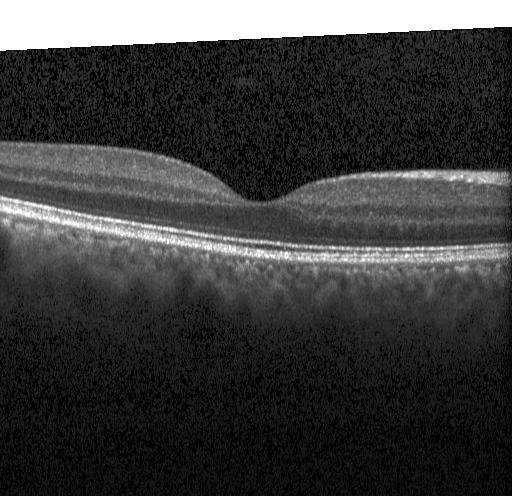 Optical coherence tomography scan; SD-OCT; macular scan; Heidelberg Spectralis OCT system. Assessment: no choroidal neovascularization, diabetic macular edema, or drusen.